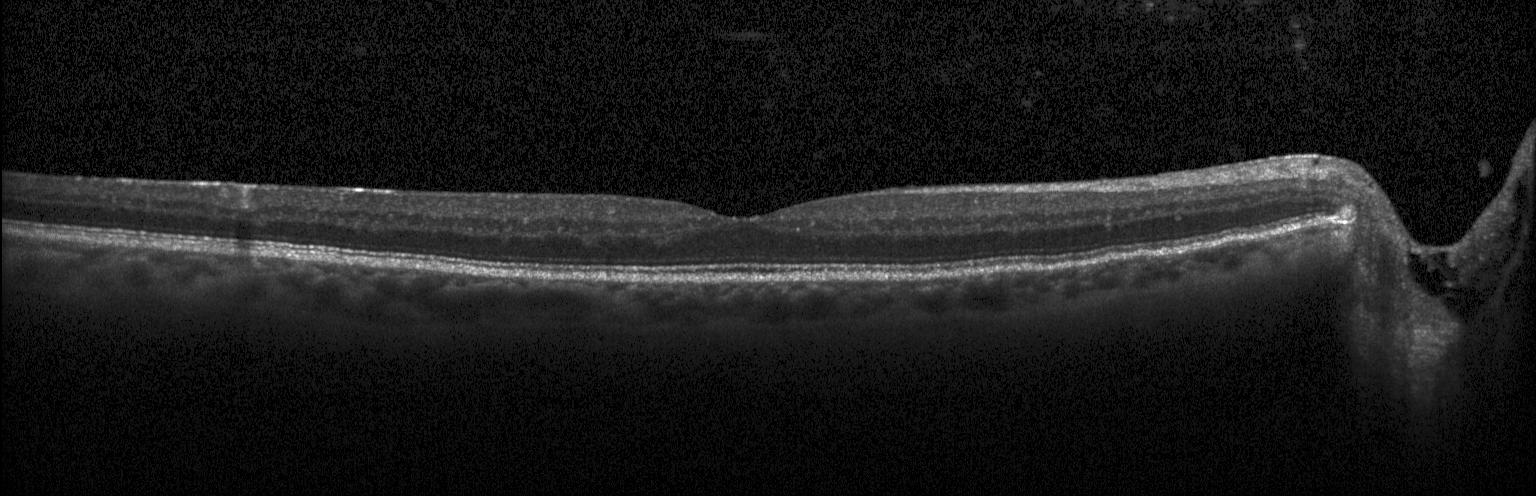 OCT B-scan · spectral-domain optical coherence tomography. The scan shows no evidence of choroidal neovascularization, diabetic macular edema, or drusen.